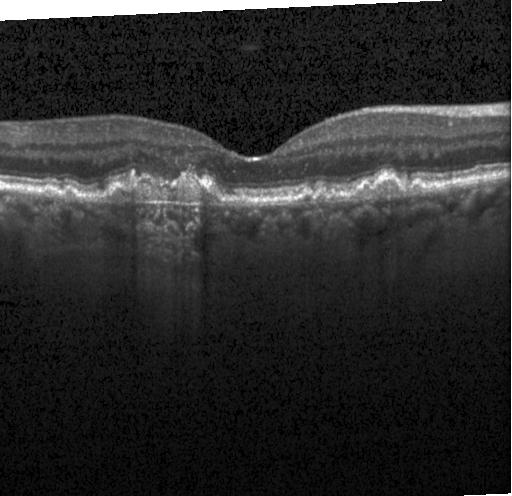
Spectral-domain OCT B-scan: a choroidal neovascular membrane.